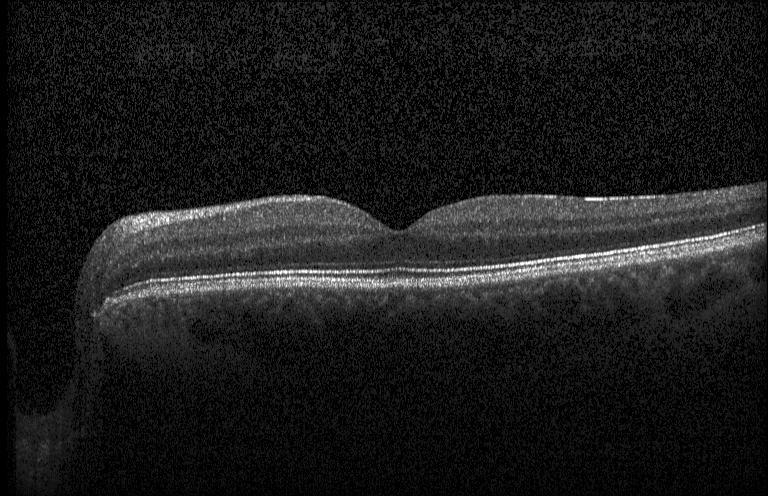
SD-OCT. Retinal OCT cross-section
Diagnosis: neither choroidal neovascularization, diabetic macular edema, nor drusen.